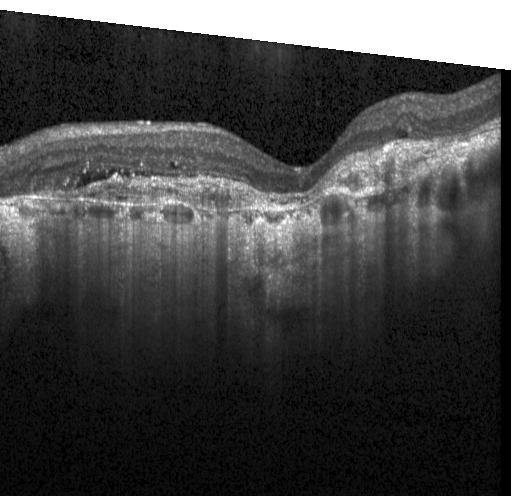
Retinal OCT cross-section showing CNV.